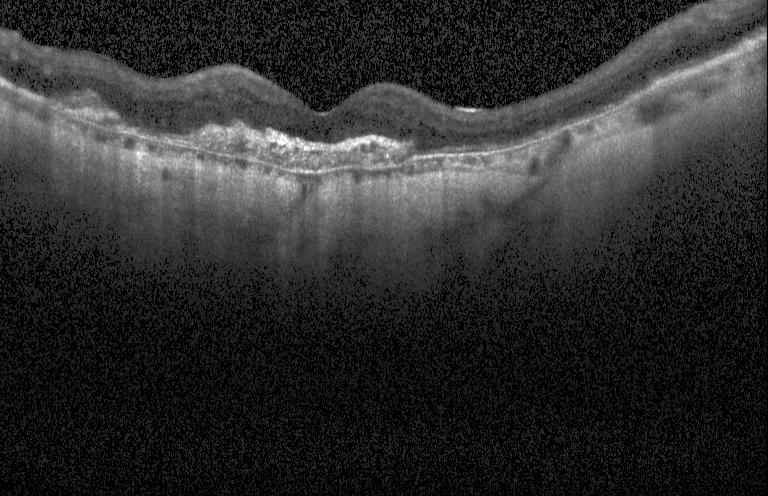
Retinal OCT B-scan. Heidelberg Spectralis OCT system. Spectral-domain OCT
Finding: a choroidal neovascular membrane.